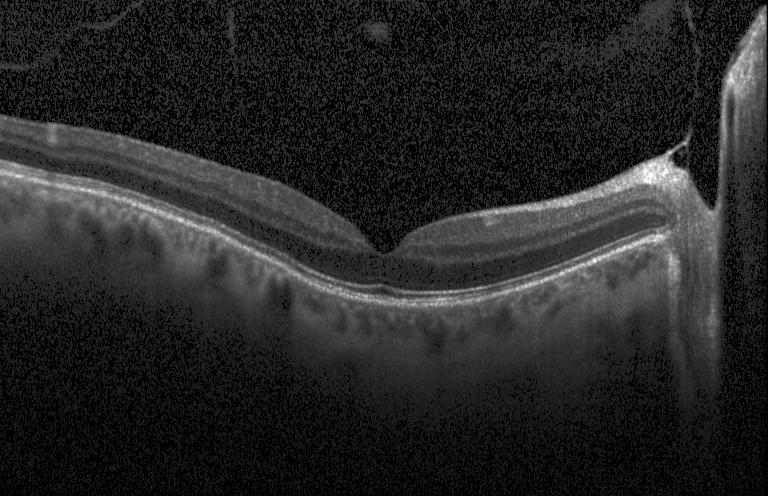
Acquired on a Heidelberg Spectralis. SD-OCT. Retinal OCT B-scan. Through the macula. The scan shows no evidence of choroidal neovascularization, diabetic macular edema, or drusen.